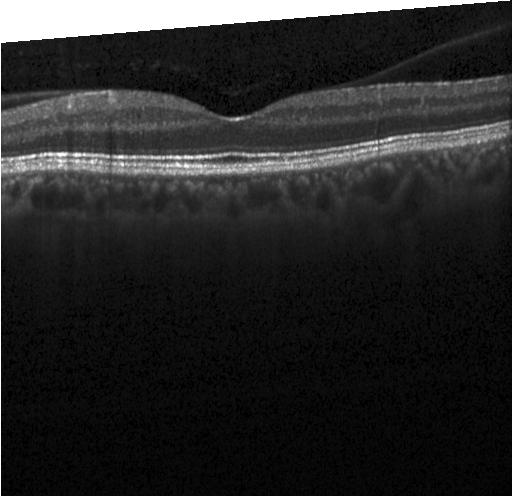 OCT B-scan showing no choroidal neovascularization, diabetic macular edema, or drusen.